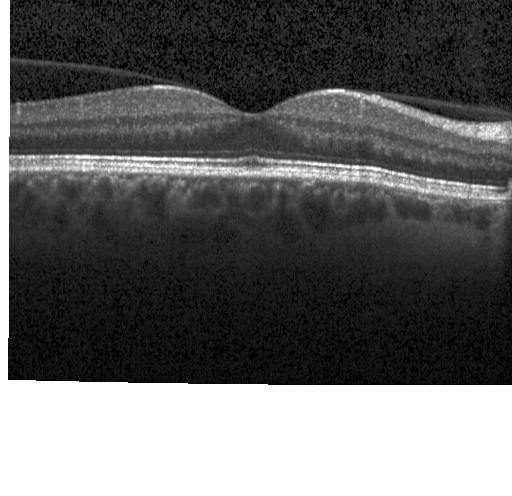
OCT B-scan; acquired on a Heidelberg Spectralis — Finding: no evidence of CNV, DME, or drusen.